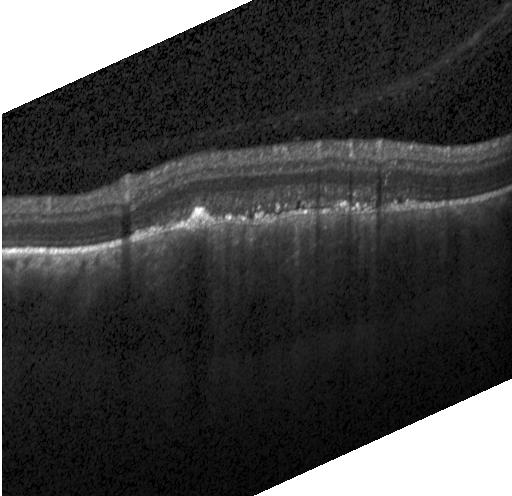
Retinal OCT cross-section
The scan shows choroidal neovascularization.